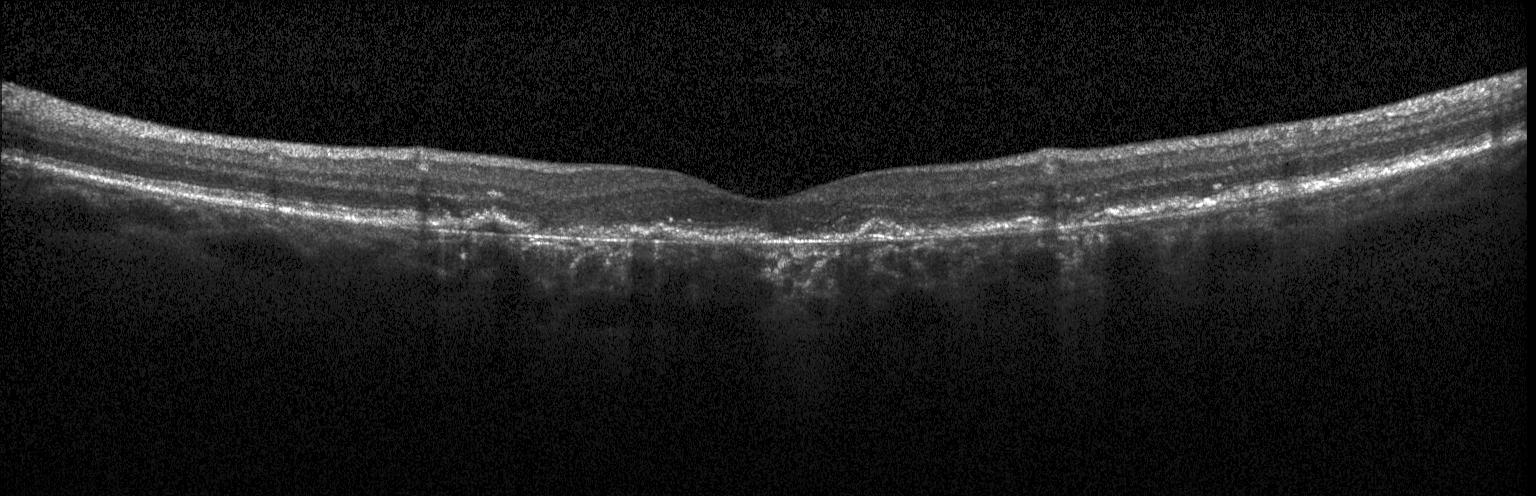 Heidelberg Spectralis. Spectral-domain optical coherence tomography. Retinal OCT B-scan — This B-scan demonstrates a choroidal neovascular membrane.